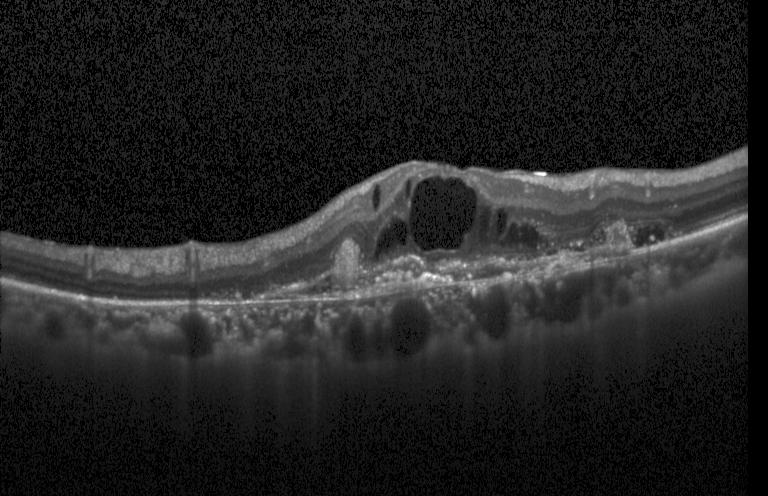 Spectral-domain OCT B-scan: CNV.